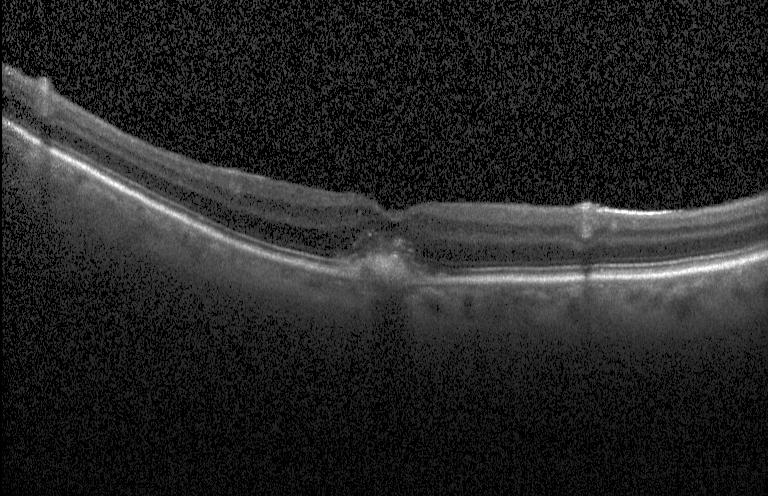

Impression: a choroidal neovascular membrane.